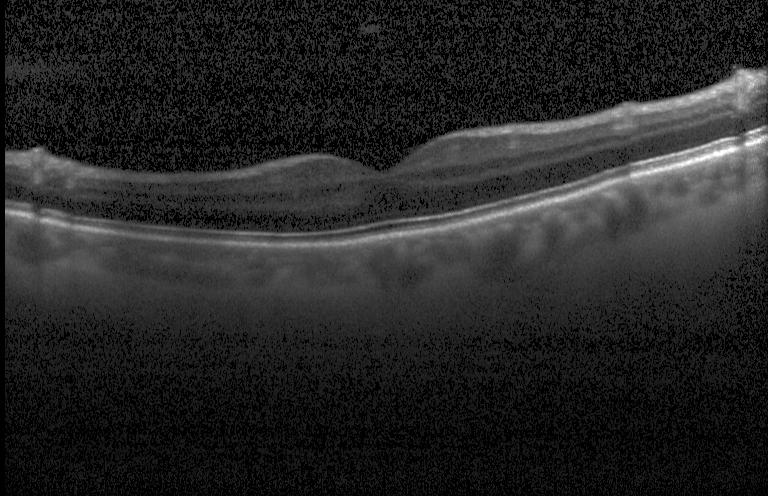 Optical coherence tomography scan; Heidelberg Spectralis; centered on the fovea
Dx: neither choroidal neovascularization, diabetic macular edema, nor drusen.